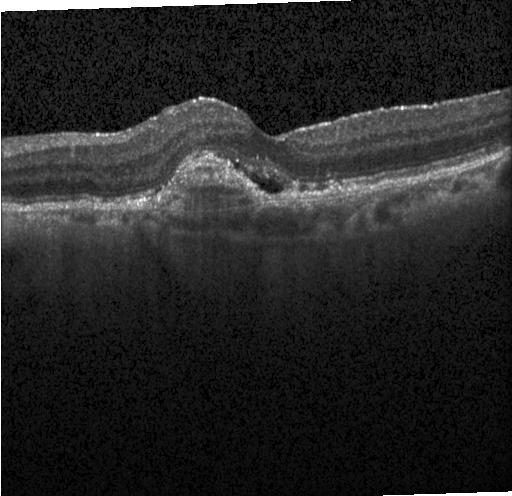

Acquired on a Heidelberg Spectralis. Centered on the fovea. OCT line scan
Finding: a choroidal neovascular membrane.